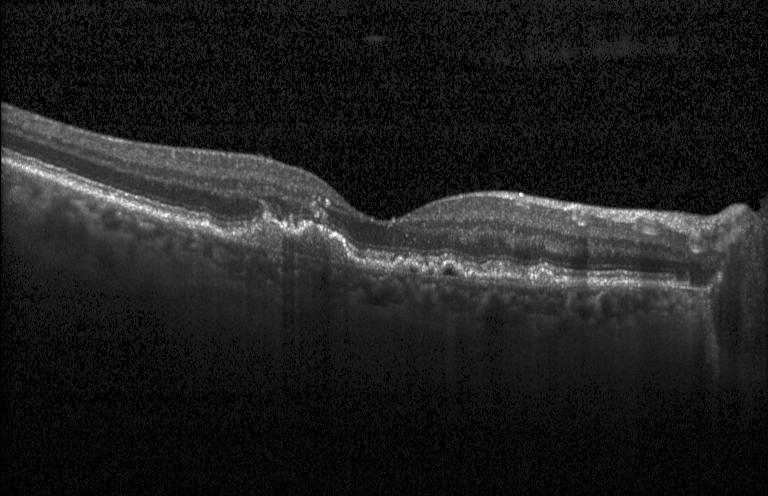 Heidelberg Spectralis, retinal OCT cross-section, spectral-domain optical coherence tomography — Impression: choroidal neovascularization.